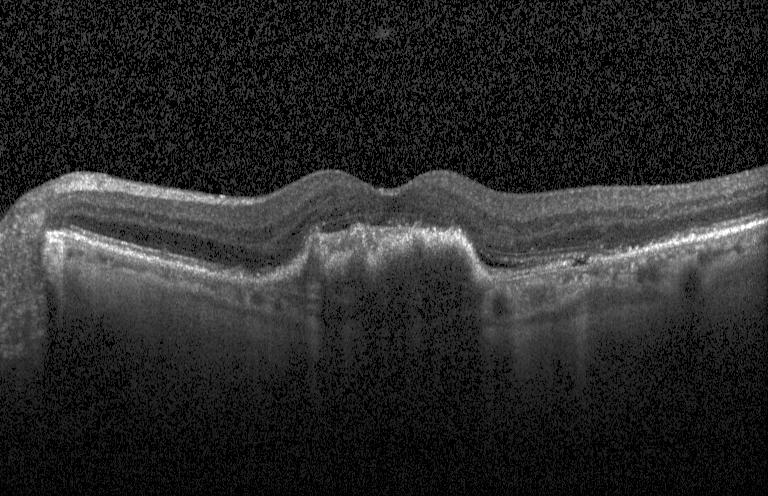

Macular OCT demonstrating CNV.